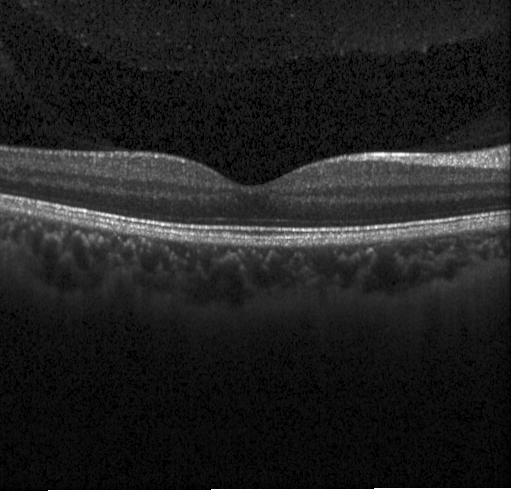
OCT finding: neither choroidal neovascularization, diabetic macular edema, nor drusen.